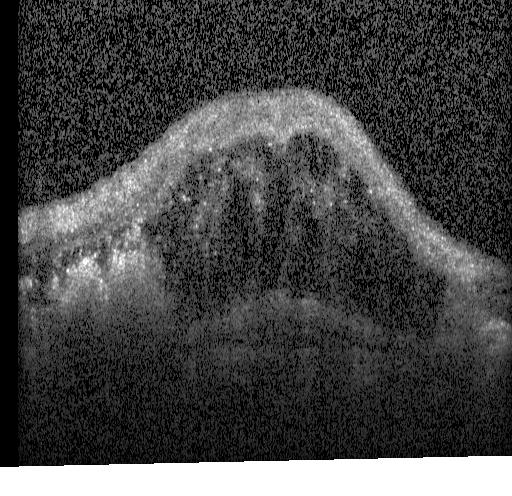
Spectral-domain OCT B-scan: DME.